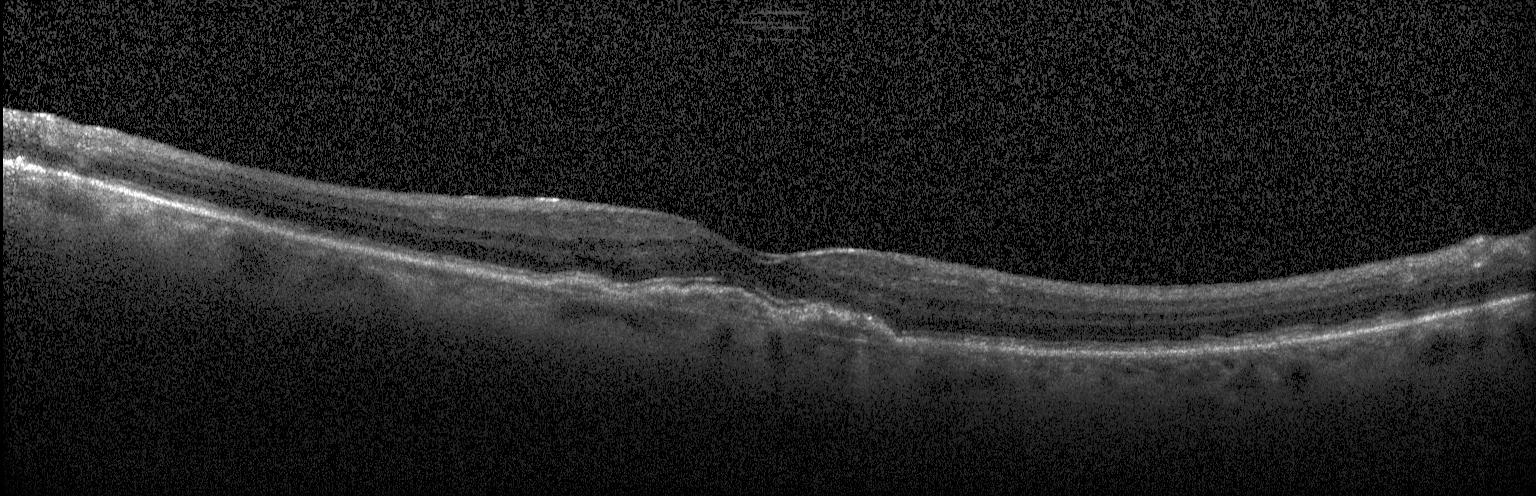

A choroidal neovascular membrane.